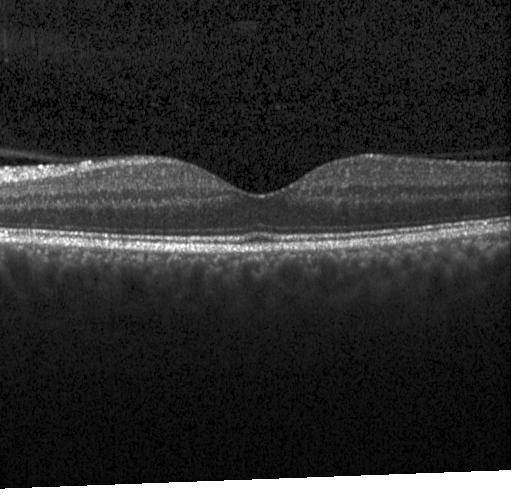

Retinal OCT B-scan · Heidelberg Spectralis · spectral-domain optical coherence tomography · horizontal scan through the fovea — Dx: no CNV, no DME, and no drusen.